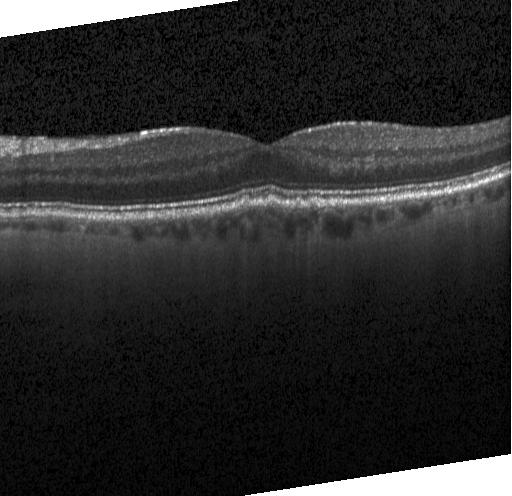
The scan shows drusen.